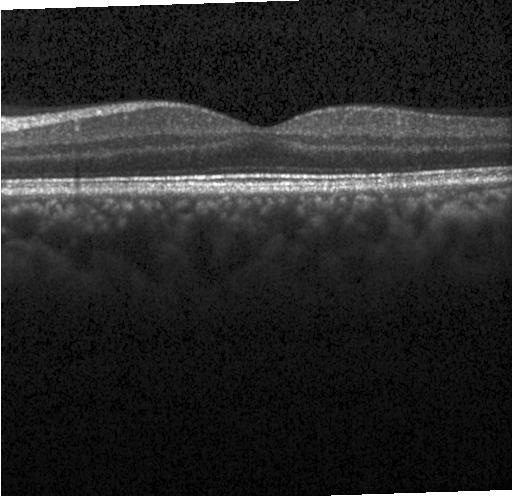 Spectral-domain optical coherence tomography; retinal OCT cross-section.
OCT finding: neither choroidal neovascularization, diabetic macular edema, nor drusen.